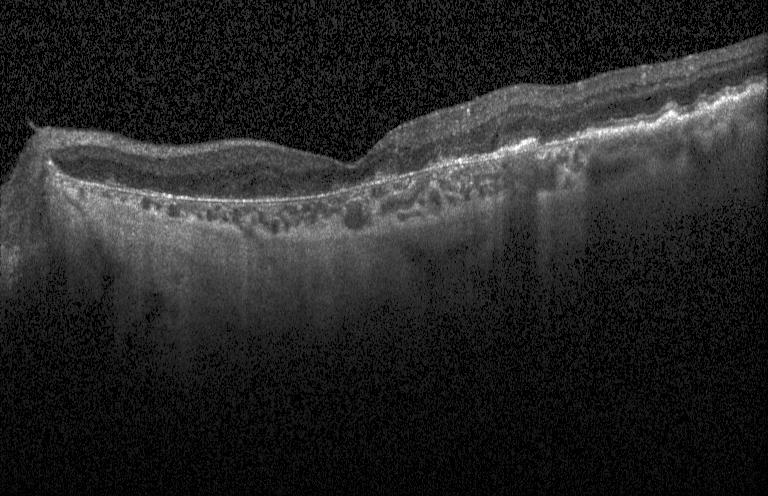
Horizontal scan through the fovea; retinal OCT cross-section
The scan shows CNV.